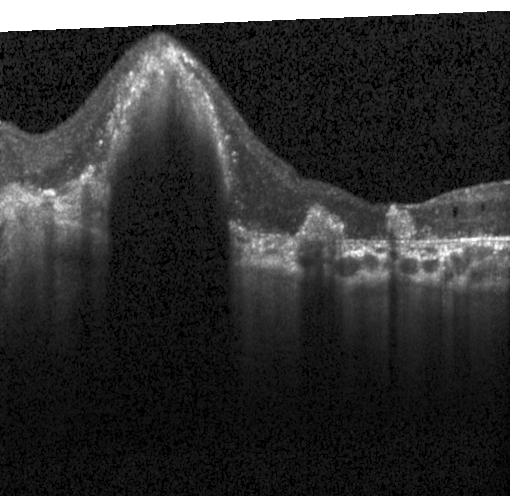 The scan shows choroidal neovascularization.